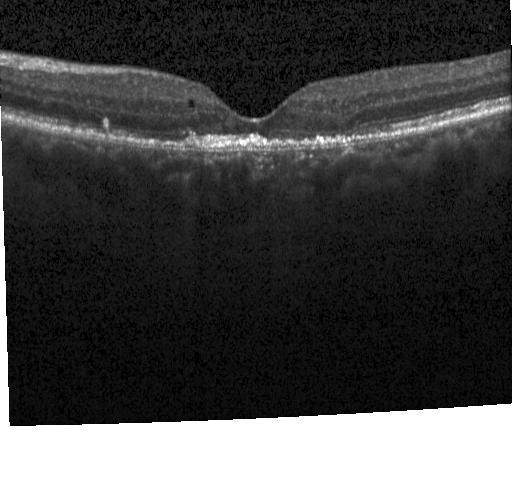

Spectral-domain optical coherence tomography · optical coherence tomography scan · centered on the fovea
Macular OCT: choroidal neovascularization (CNV).